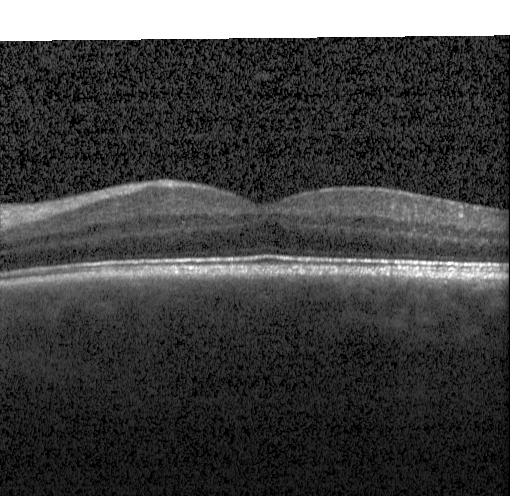
Instrument: Heidelberg Spectralis, through the macula, optical coherence tomography B-scan.
Dx: no choroidal neovascularization, no diabetic macular edema, and no drusen.